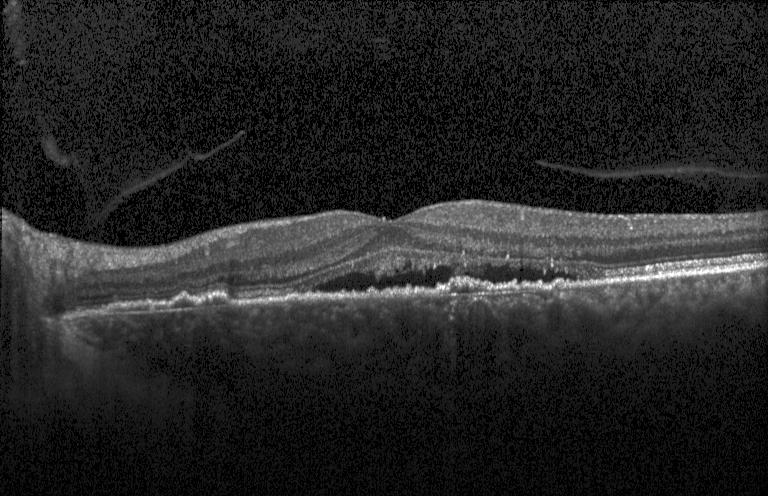

Spectral-domain OCT B-scan: choroidal neovascularization.